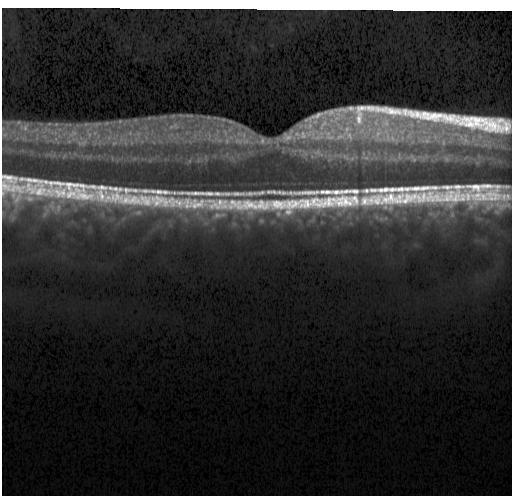

Horizontal scan through the fovea. Optical coherence tomography B-scan. Heidelberg Spectralis OCT system. Spectral-domain optical coherence tomography. Neither CNV, DME, nor drusen.